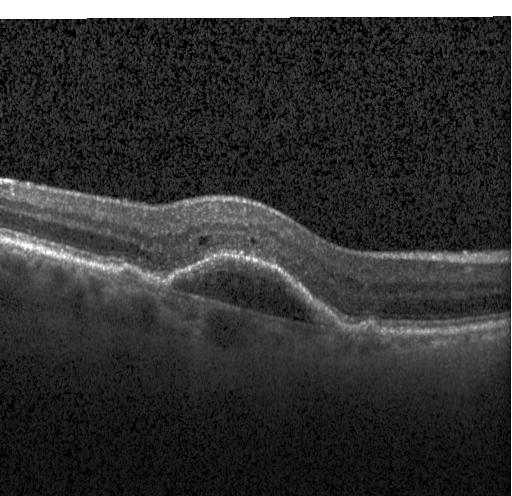
Assessment: choroidal neovascularization.